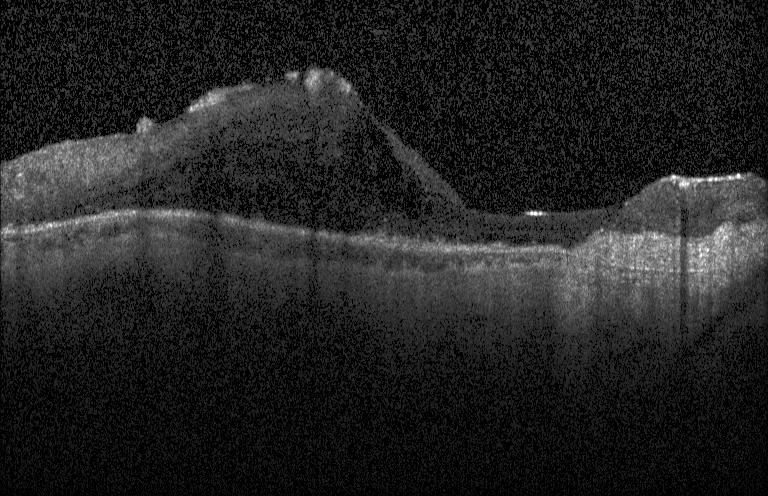
SD-OCT, acquired on a Heidelberg Spectralis, OCT line scan
Diagnosis: DME.